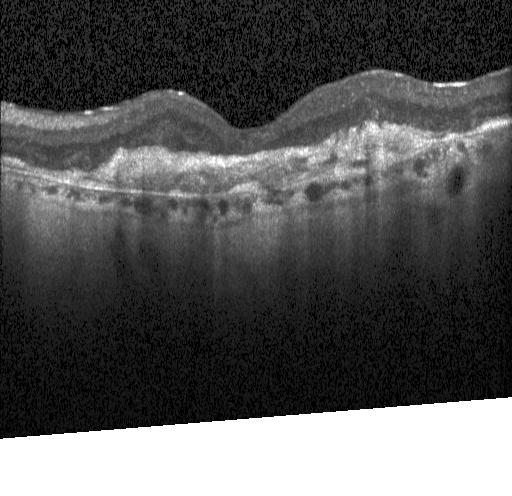
OCT line scan; through the macula
Finding: a choroidal neovascular membrane.